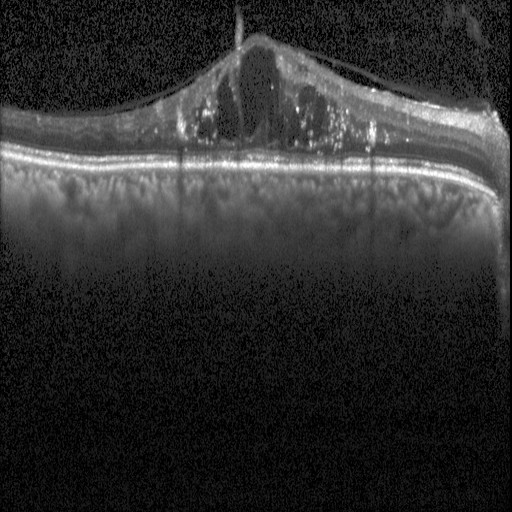 Optical coherence tomography B-scan; Heidelberg Spectralis; through the macula; spectral-domain optical coherence tomography
Macular OCT: diabetic macular edema (DME).